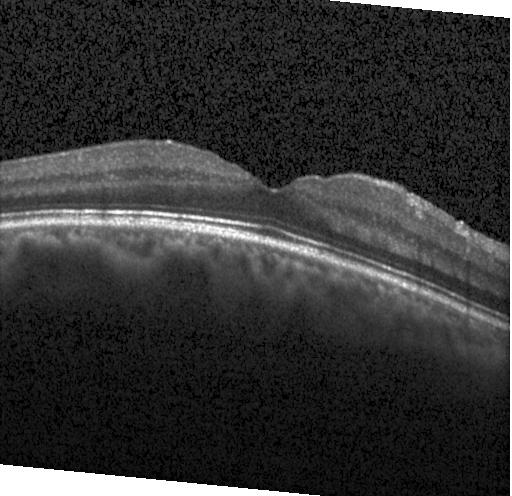 The scan shows no choroidal neovascularization, no diabetic macular edema, and no drusen.